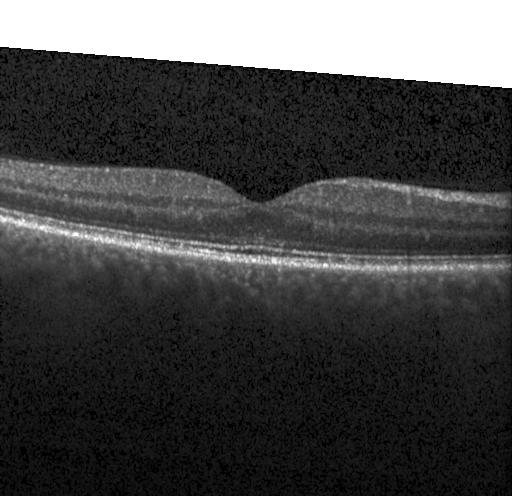 Diagnosis: no evidence of choroidal neovascularization, diabetic macular edema, or drusen.